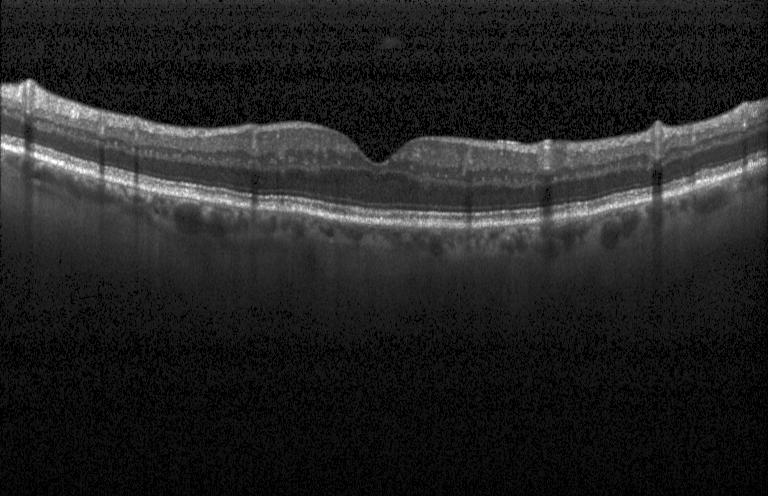
OCT line scan
Finding: no choroidal neovascularization, diabetic macular edema, or drusen.